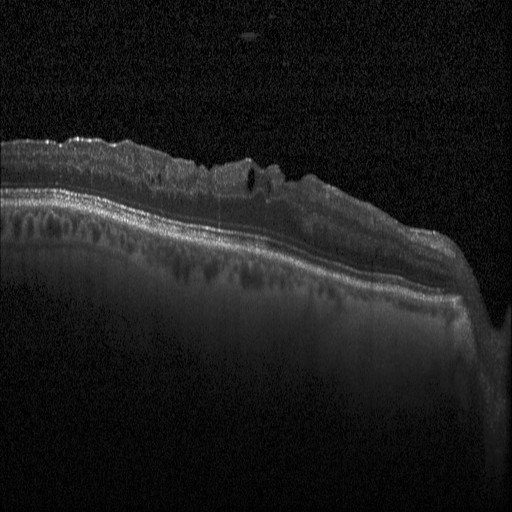

Impression: DME.